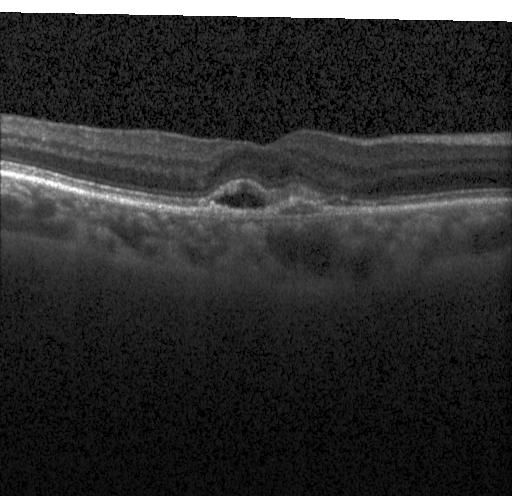
The scan shows a choroidal neovascular membrane.